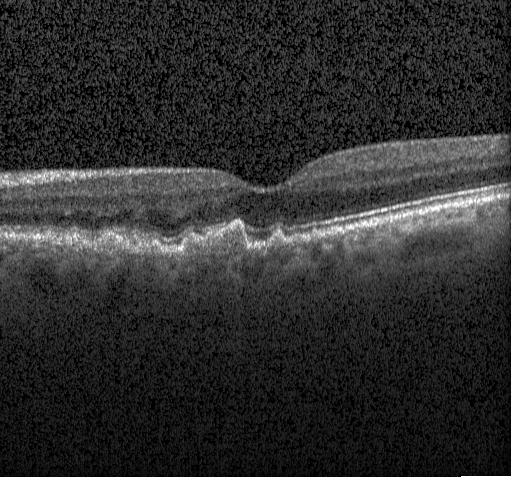

OCT line scan.
OCT finding: sub-RPE drusenoid deposits.